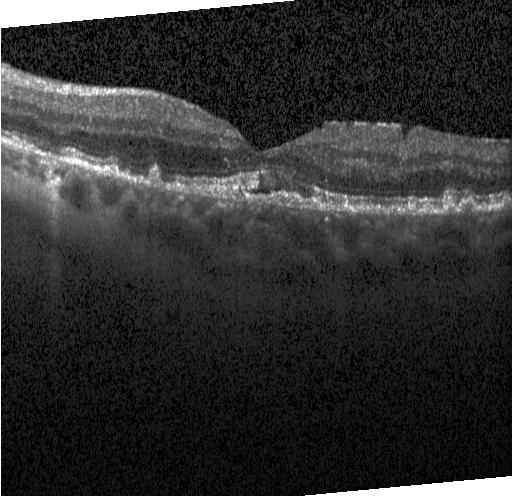 Acquired on a Heidelberg Spectralis, OCT line scan.
Impression: choroidal neovascularization (CNV).